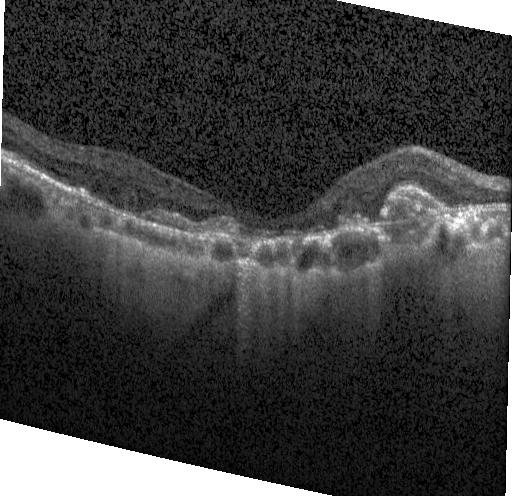

SD-OCT · instrument: Heidelberg Spectralis · retinal OCT B-scan.
Impression: a choroidal neovascular membrane.